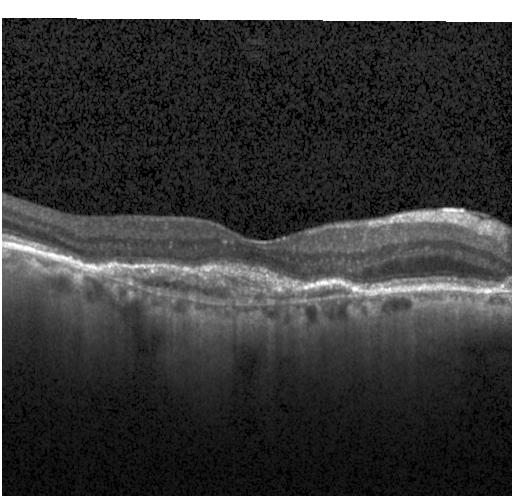 Spectral-domain optical coherence tomography; optical coherence tomography B-scan
Impression: choroidal neovascularization.